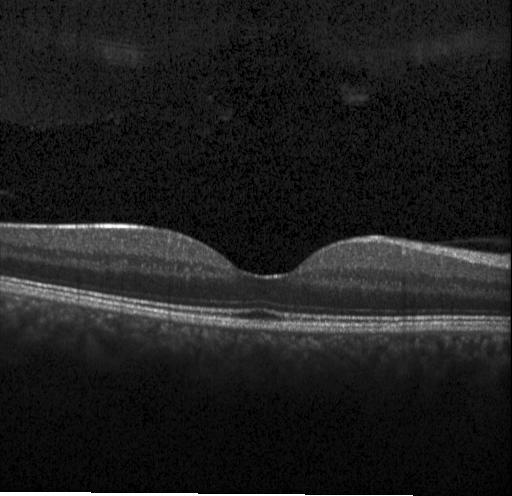
Acquired on a Heidelberg Spectralis · retinal OCT cross-section · fovea-centered
Dx: no evidence of choroidal neovascularization, diabetic macular edema, or drusen.